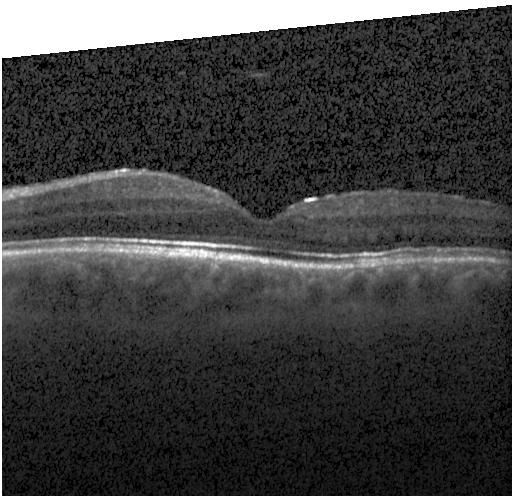 Diagnosis: no CNV, DME, or drusen.